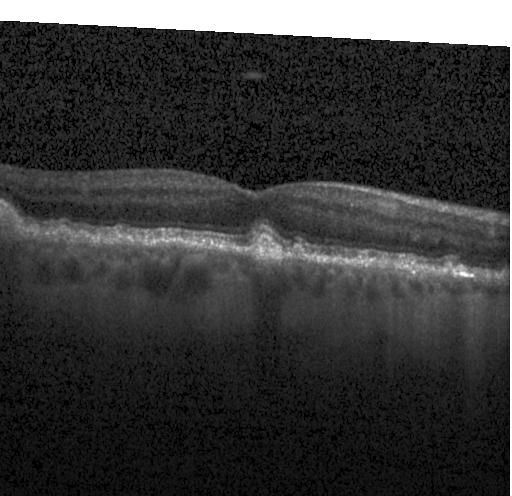

Finding: multiple drusen.